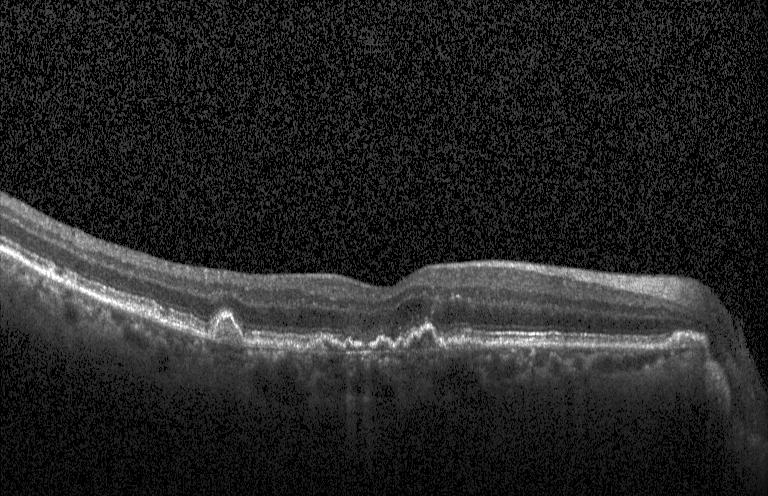
Diagnosis: drusen.